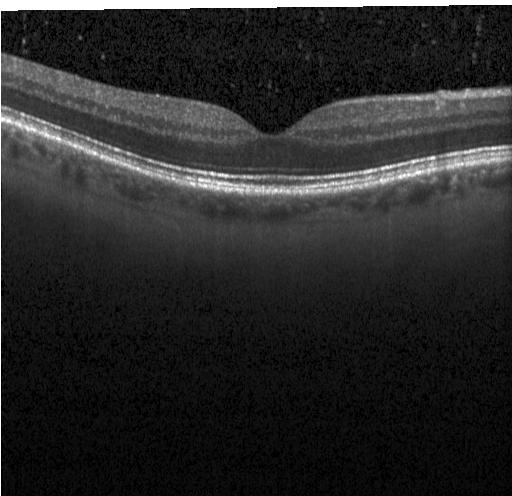 Diagnosis: no evidence of choroidal neovascularization, diabetic macular edema, or drusen.